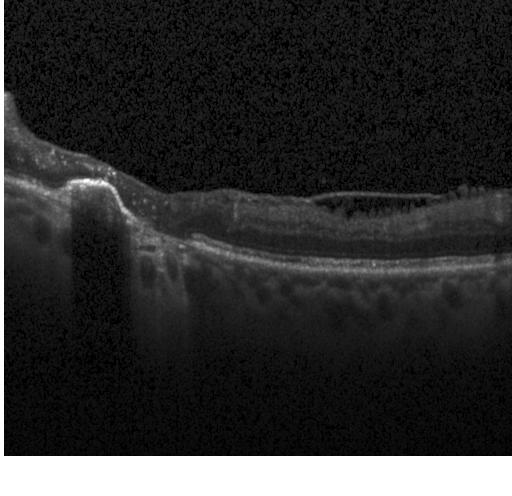

This B-scan demonstrates a choroidal neovascular membrane.